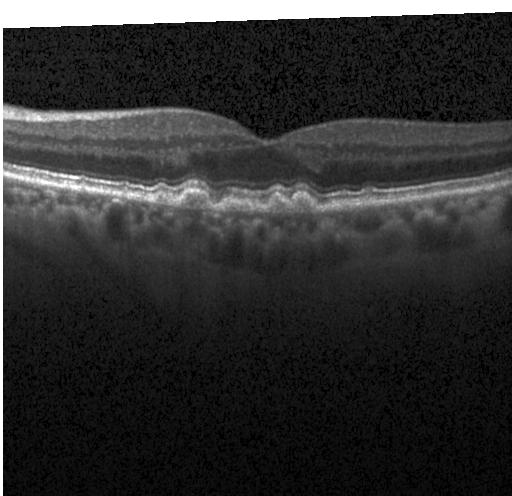

Finding: drusen.